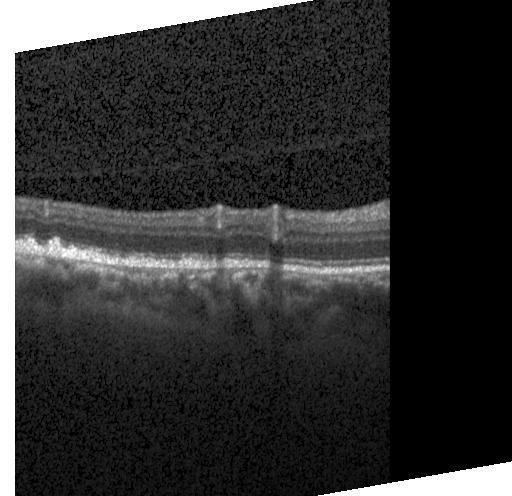

This B-scan demonstrates drusen.